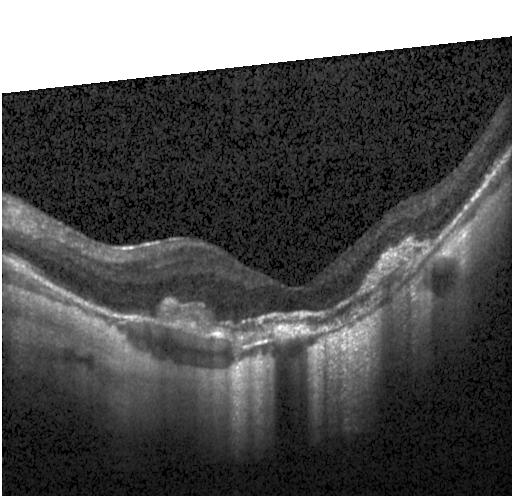

OCT B-scan showing a choroidal neovascular membrane.